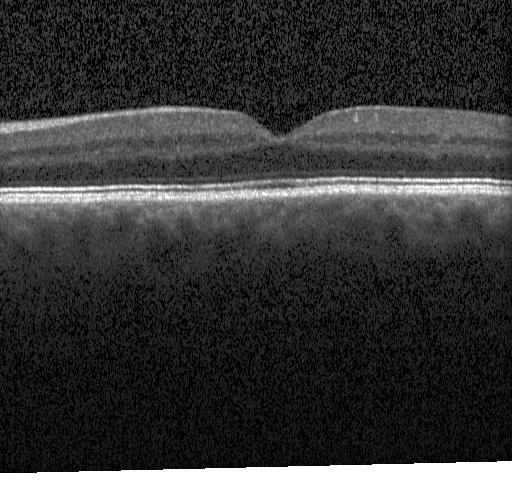
Retinal OCT B-scan; centered on the fovea — Finding: no choroidal neovascularization, diabetic macular edema, or drusen.